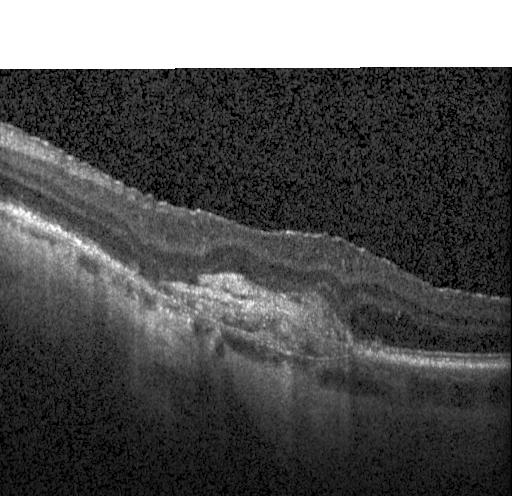 OCT B-scan showing a choroidal neovascular membrane.